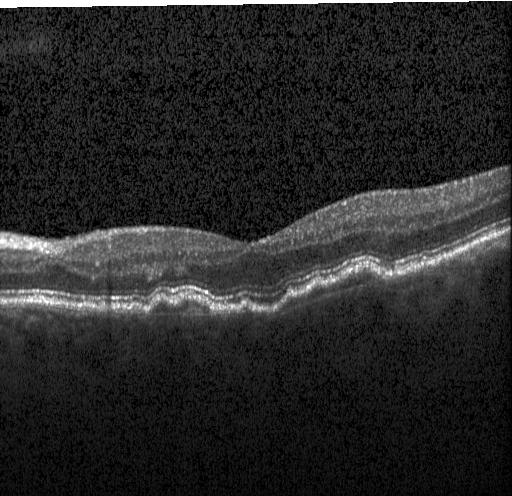 Fovea-centered · optical coherence tomography B-scan · spectral-domain optical coherence tomography · instrument: Heidelberg Spectralis
Finding: a choroidal neovascular membrane.